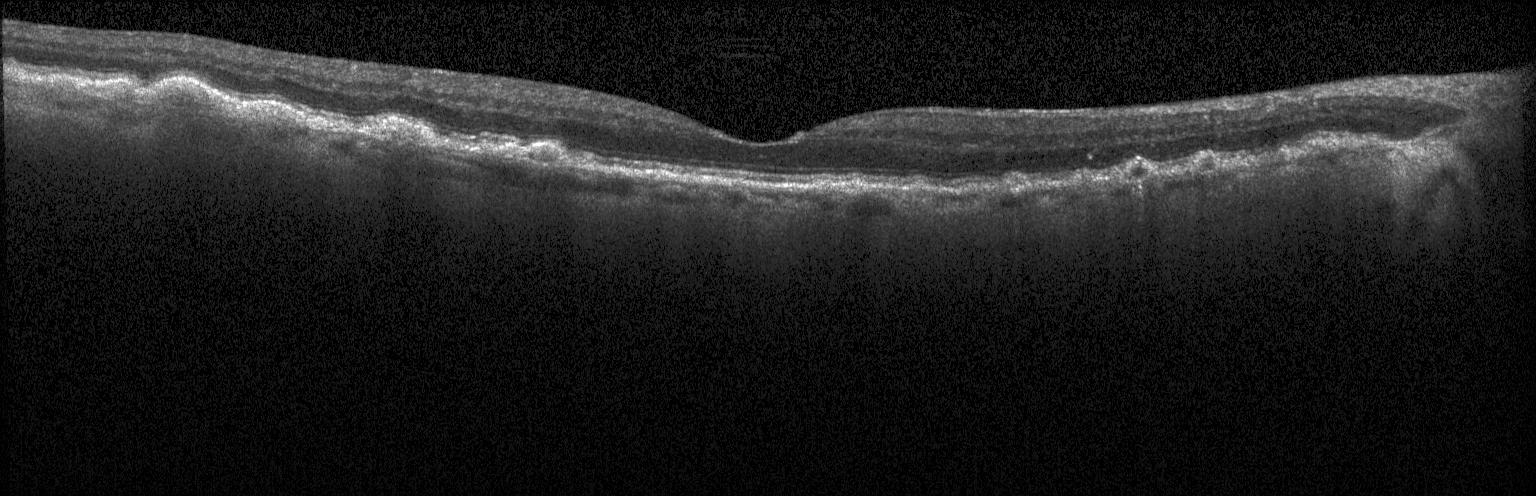
Multiple drusen.